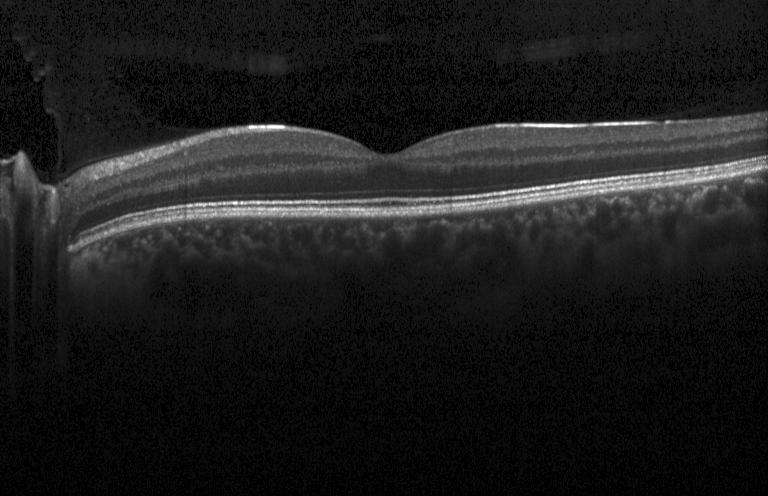
Optical coherence tomography scan.
Diagnosis: neither CNV, DME, nor drusen.